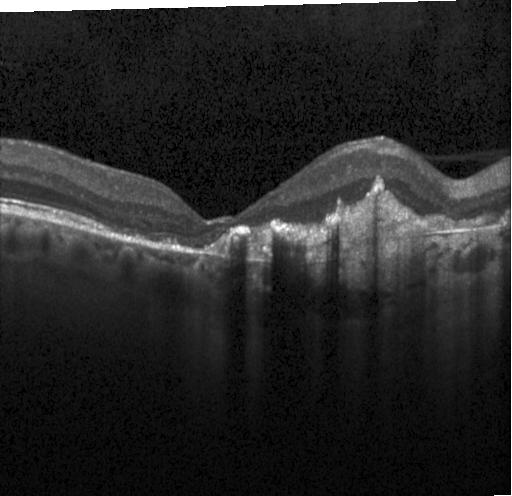 Through the macula; Heidelberg Spectralis OCT system; optical coherence tomography B-scan.
Impression: CNV.